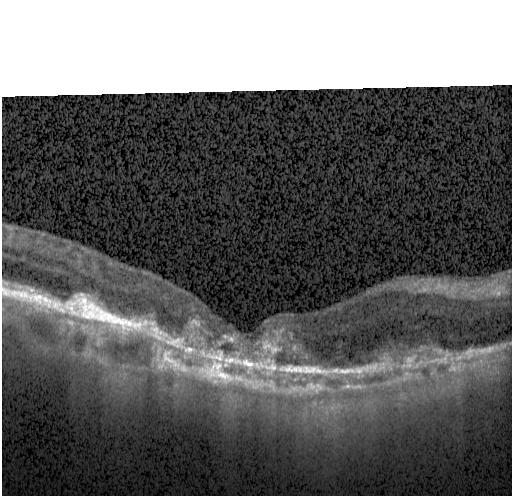
Macular scan. Optical coherence tomography scan — Finding: CNV.